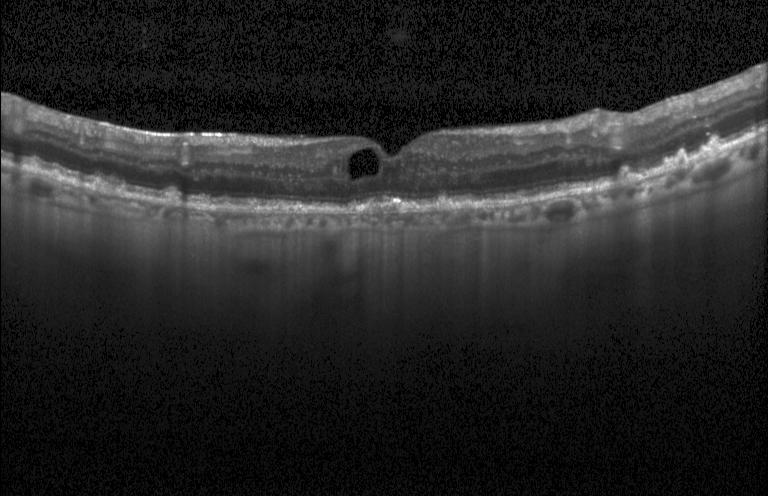
Retinal OCT B-scan
Dx: a choroidal neovascular membrane.